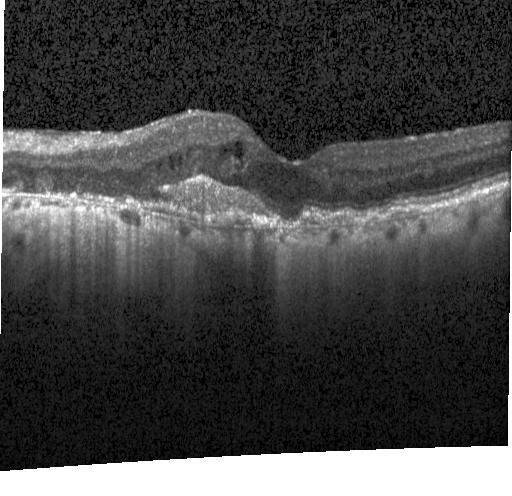 Fovea-centered; OCT line scan; SD-OCT; Heidelberg Spectralis. The scan shows a choroidal neovascular membrane.